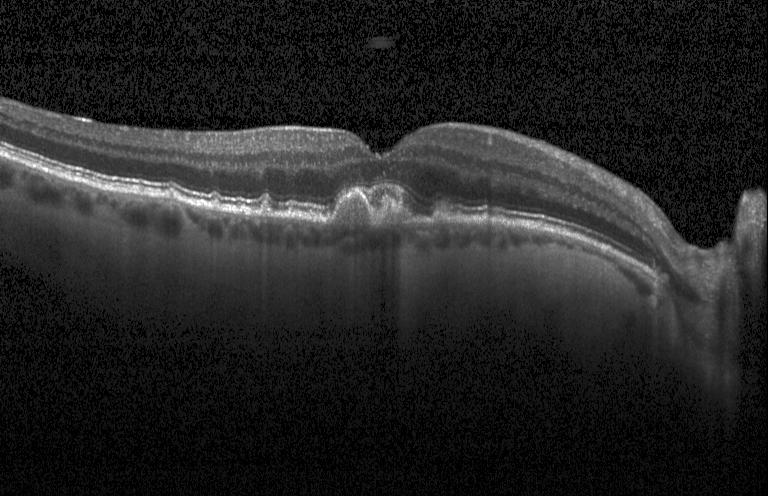
Instrument: Heidelberg Spectralis, OCT line scan, fovea-centered
Dx: multiple drusen.